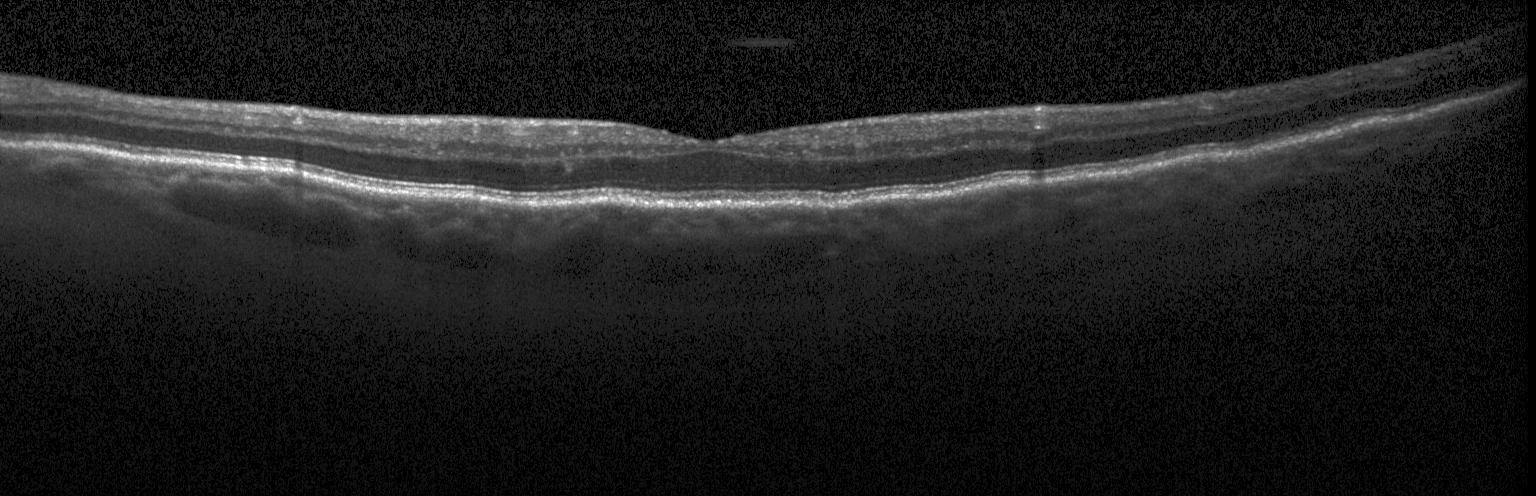 Heidelberg Spectralis, optical coherence tomography B-scan. No evidence of choroidal neovascularization, diabetic macular edema, or drusen.